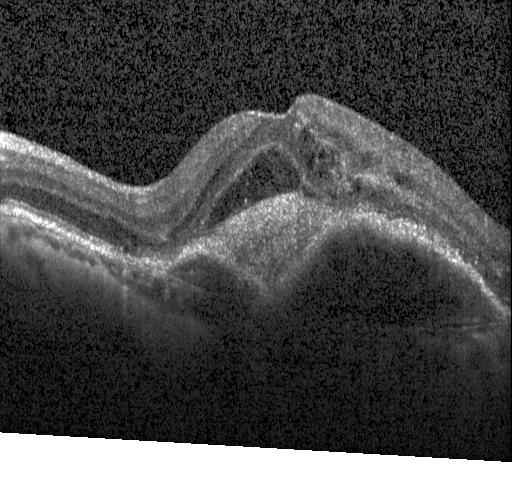 Horizontal scan through the fovea, Heidelberg Spectralis OCT system, optical coherence tomography scan
Choroidal neovascularization.